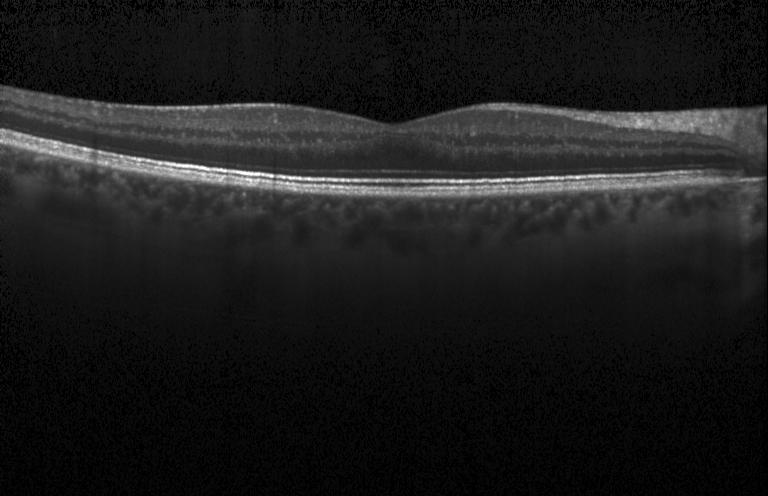
The scan shows no choroidal neovascularization, no diabetic macular edema, and no drusen.